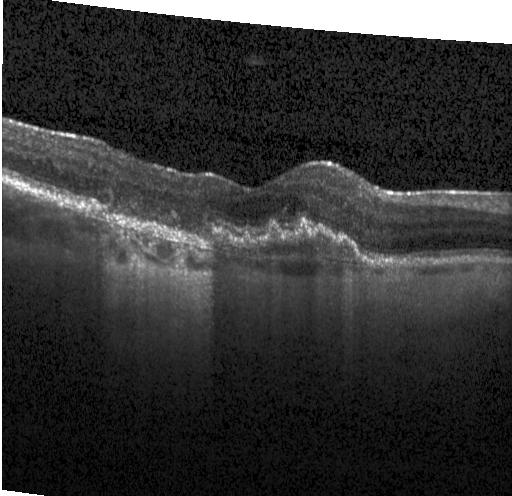 Assessment: choroidal neovascularization (CNV).